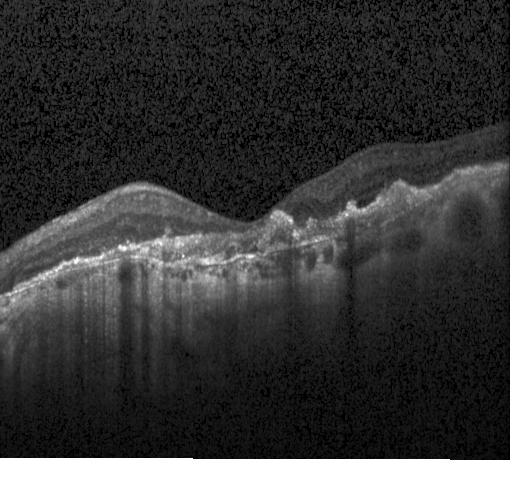

Macular OCT: choroidal neovascularization.